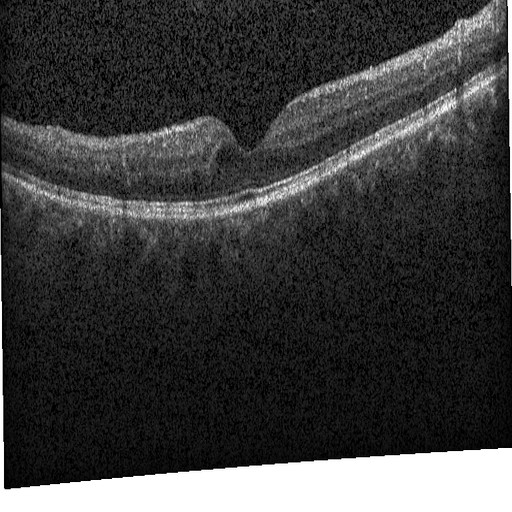 OCT scan showing DME.